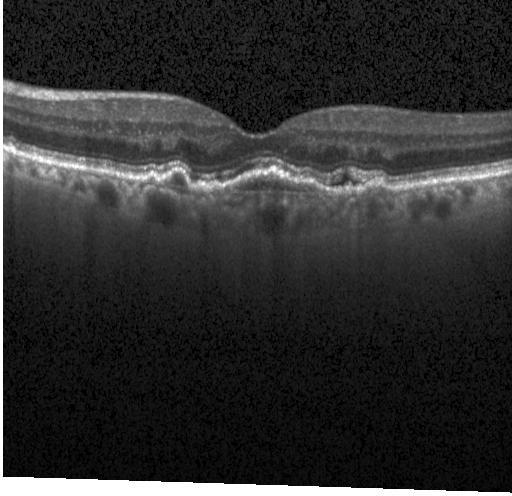 Impression: CNV.